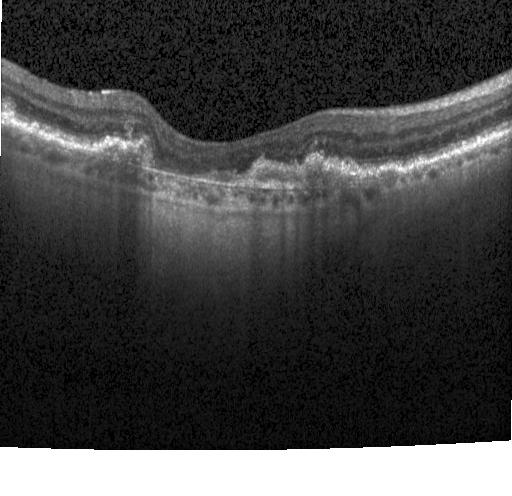
Impression: a choroidal neovascular membrane.